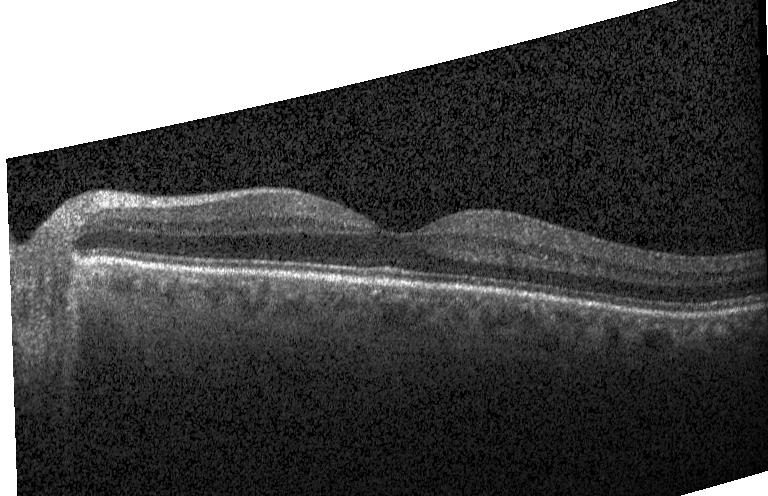
Diagnosis: neither CNV, DME, nor drusen.